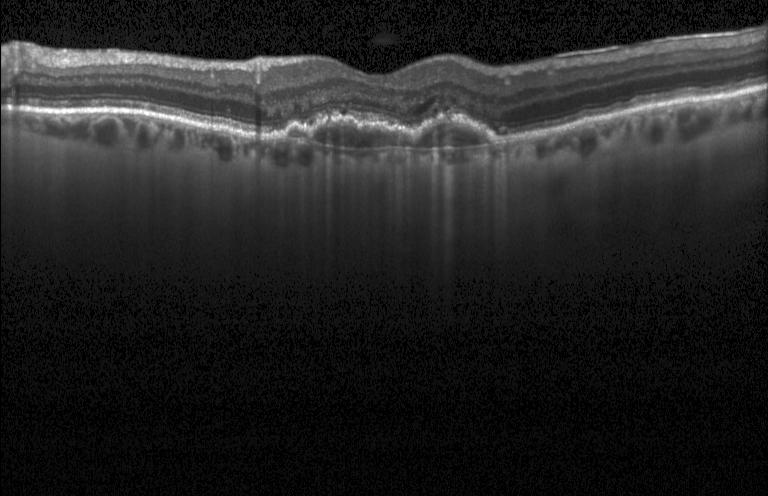
SD-OCT. Acquired on a Heidelberg Spectralis. Retinal OCT B-scan. Fovea-centered. Assessment: choroidal neovascularization.